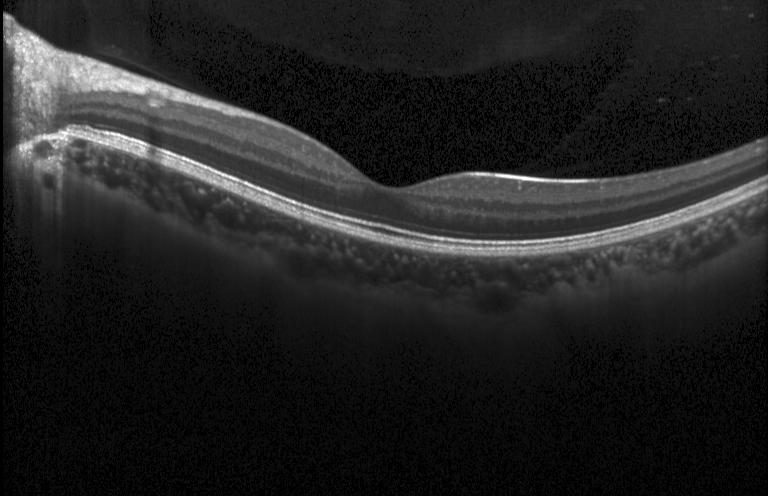 Spectral-domain OCT. Heidelberg Spectralis OCT system. OCT B-scan
The scan shows no evidence of choroidal neovascularization, diabetic macular edema, or drusen.